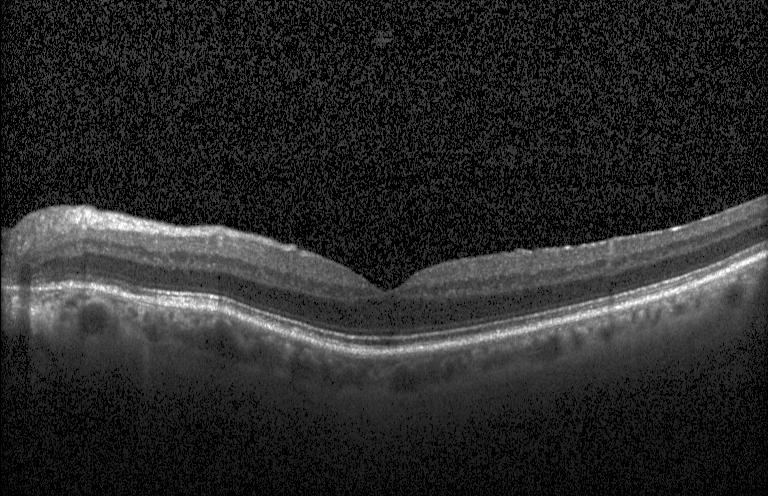
Finding: no evidence of CNV, DME, or drusen.